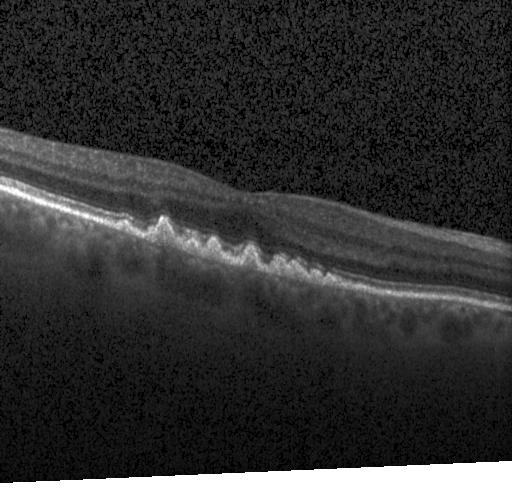 Fovea-centered · OCT line scan. This B-scan demonstrates sub-RPE drusenoid deposits.